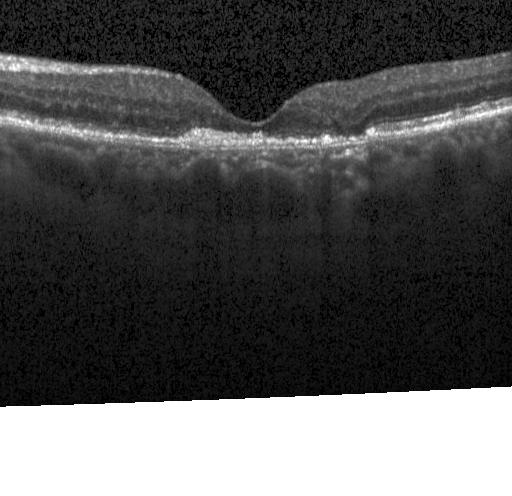

OCT finding: CNV.